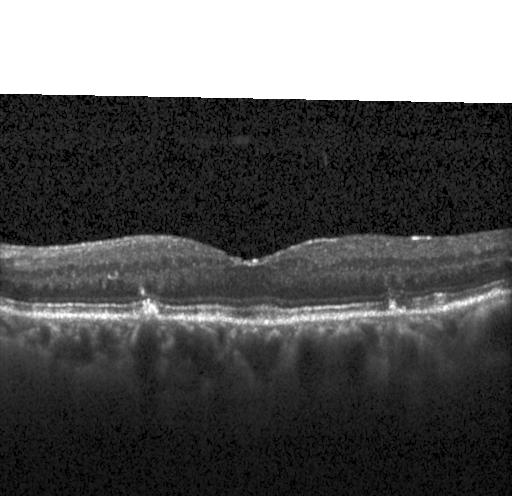
Retinal OCT B-scan. Impression: sub-RPE drusenoid deposits.